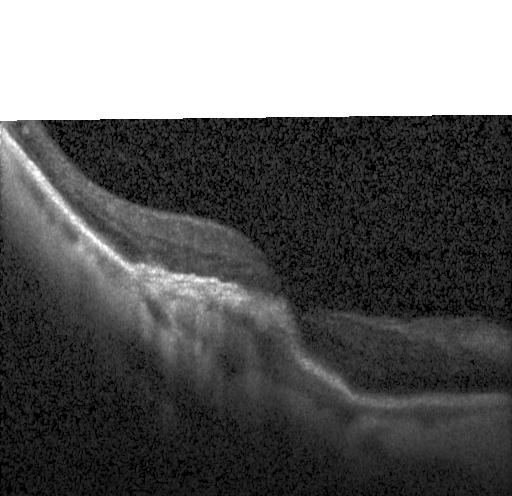 Diagnosis: choroidal neovascularization (CNV).